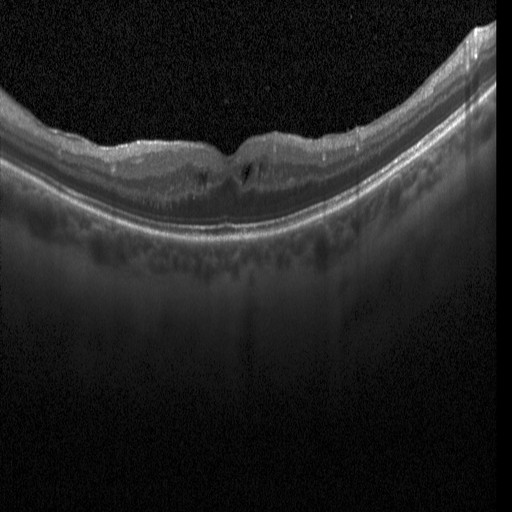 Optical coherence tomography scan
Finding: diabetic macular edema.